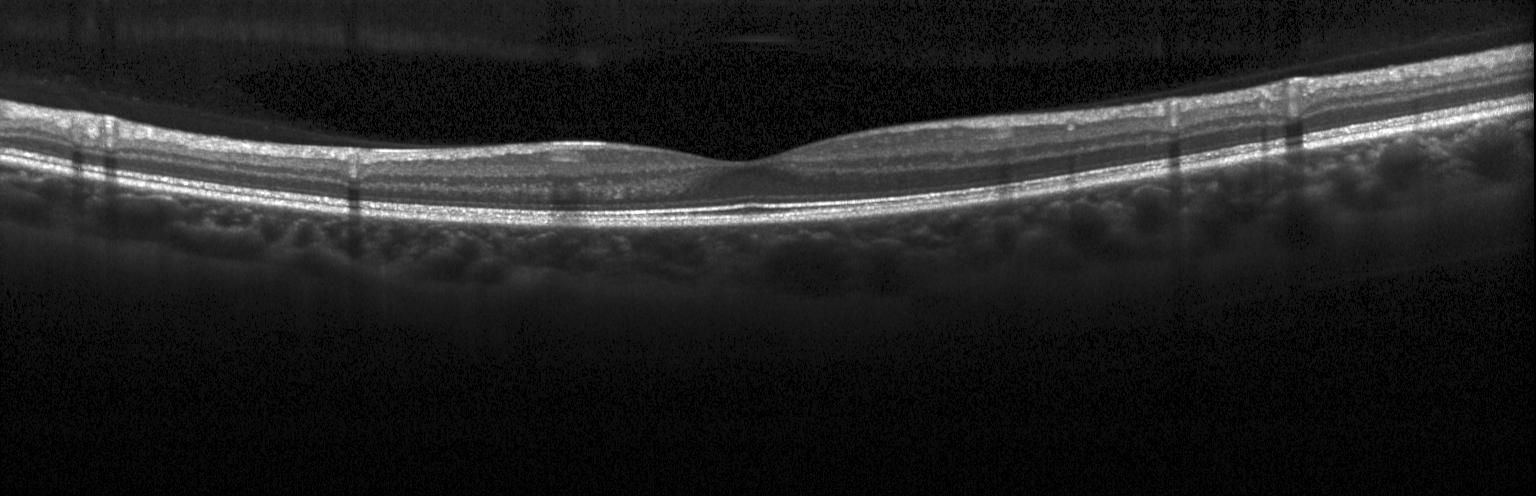 Heidelberg Spectralis, OCT line scan, spectral-domain optical coherence tomography, centered on the fovea
Assessment: no evidence of CNV, DME, or drusen.